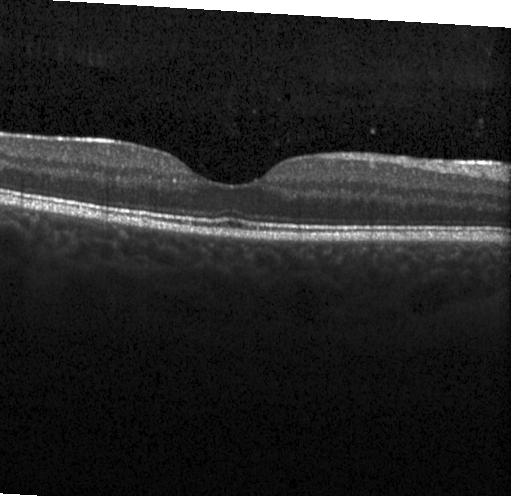 Instrument: Heidelberg Spectralis; OCT B-scan
No choroidal neovascularization, diabetic macular edema, or drusen.